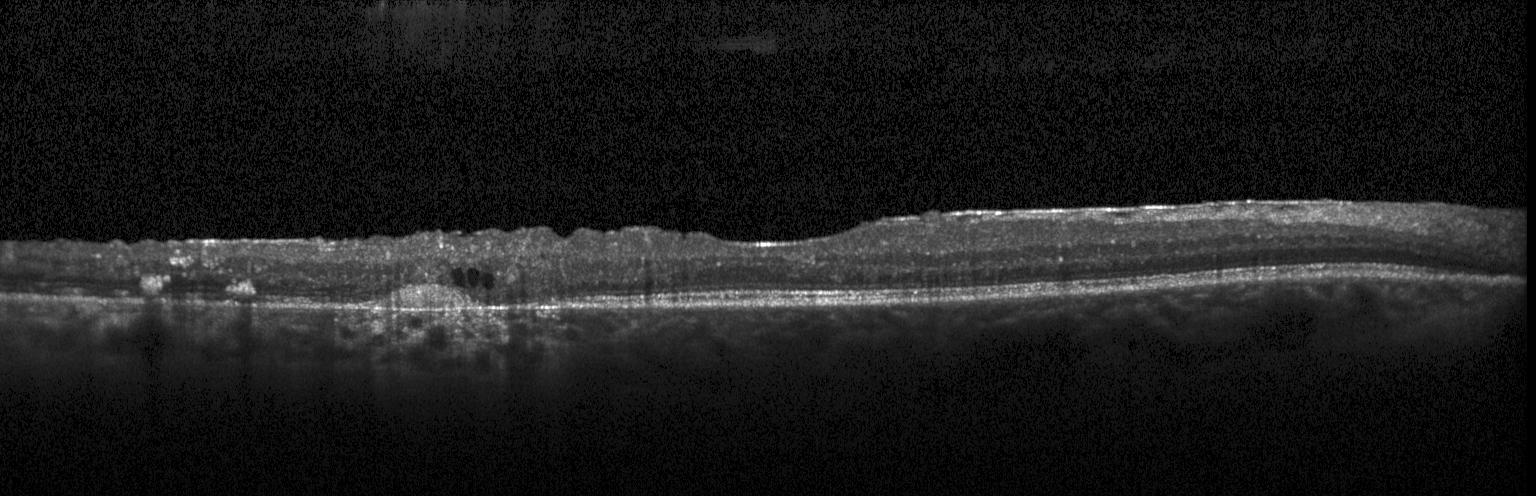

Heidelberg Spectralis, macular scan, spectral-domain optical coherence tomography, optical coherence tomography scan — Impression: choroidal neovascularization (CNV).